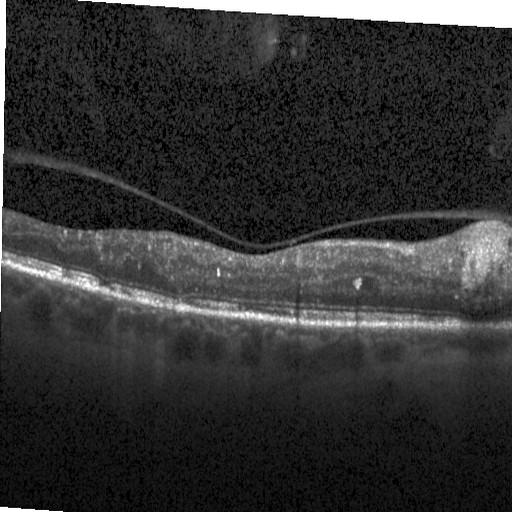

Optical coherence tomography scan
Diagnosis: diabetic macular edema (DME).